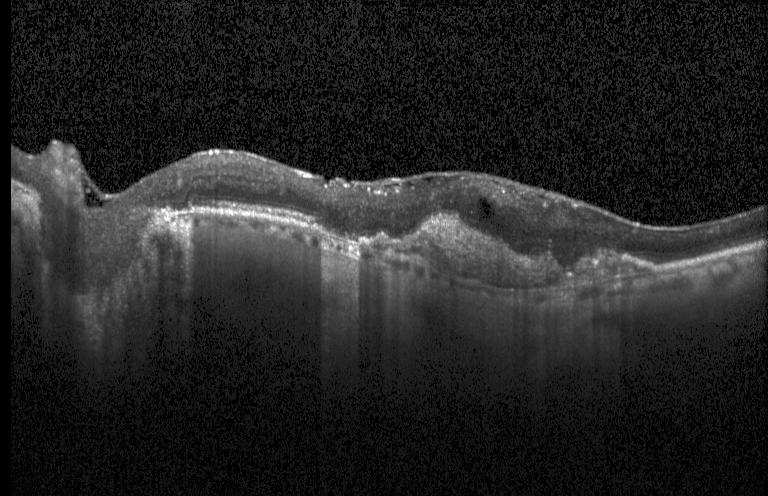

OCT line scan. SD-OCT
A choroidal neovascular membrane.